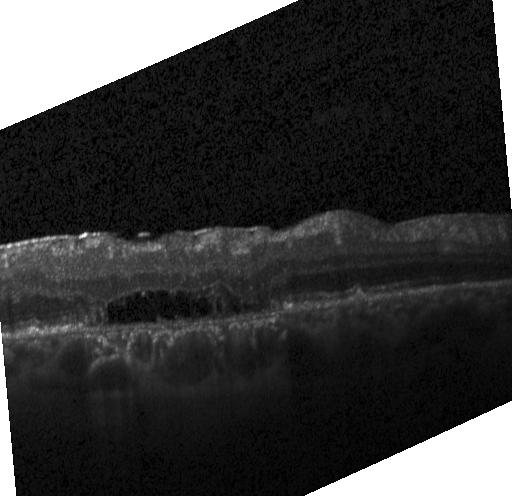

Spectral-domain OCT; OCT line scan; acquired on a Heidelberg Spectralis; horizontal scan through the fovea — Finding: choroidal neovascularization (CNV).